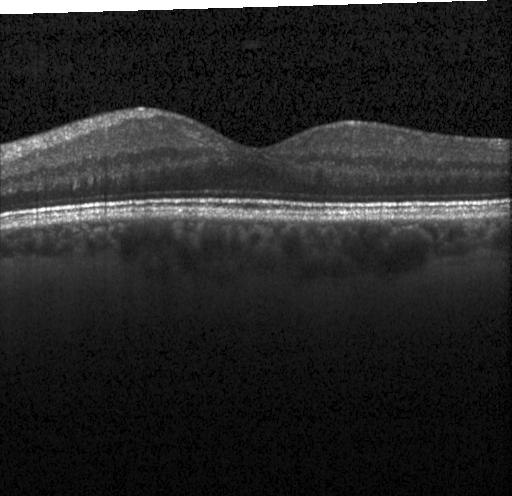 Macular OCT: no evidence of choroidal neovascularization, diabetic macular edema, or drusen.